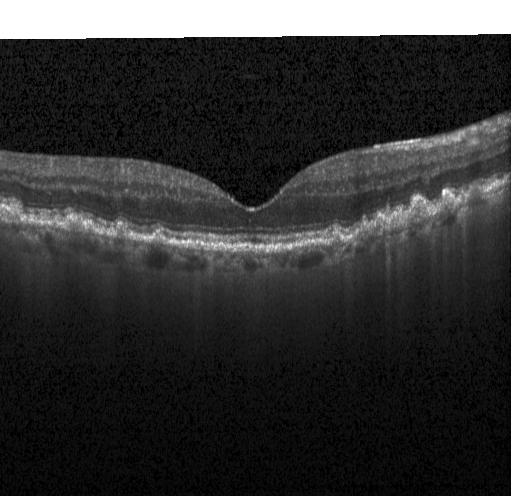

Heidelberg Spectralis · retinal OCT cross-section.
Dx: sub-RPE drusenoid deposits.